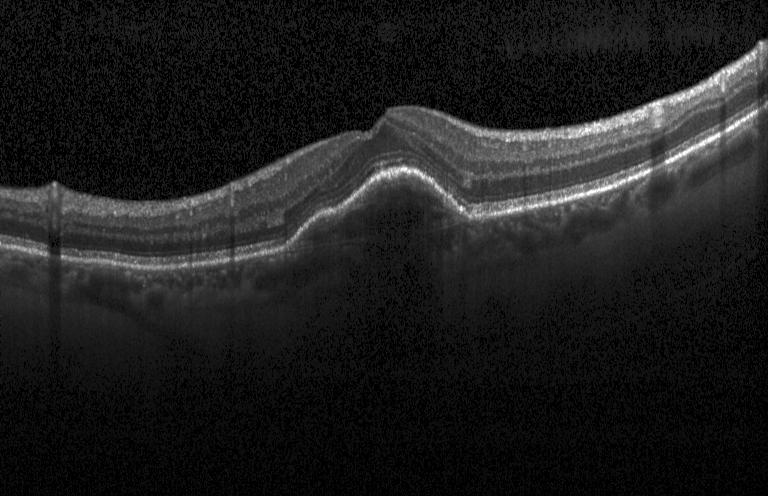
Optical coherence tomography B-scan.
This B-scan demonstrates a choroidal neovascular membrane.